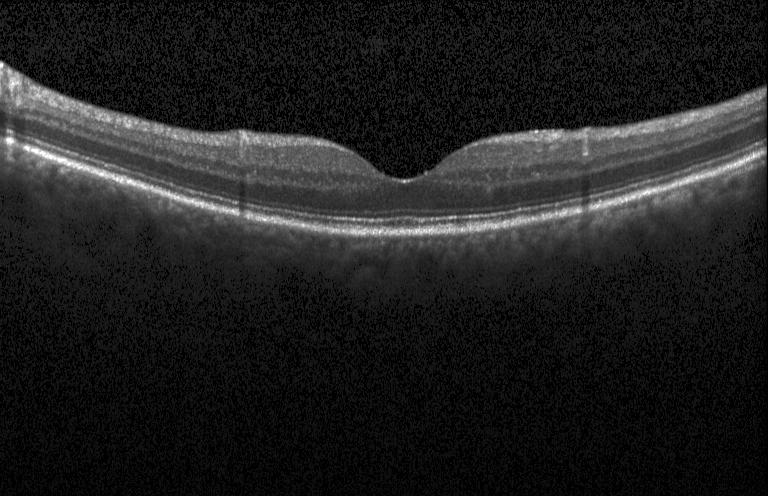

SD-OCT. Retinal OCT cross-section
Finding: no choroidal neovascularization, diabetic macular edema, or drusen.